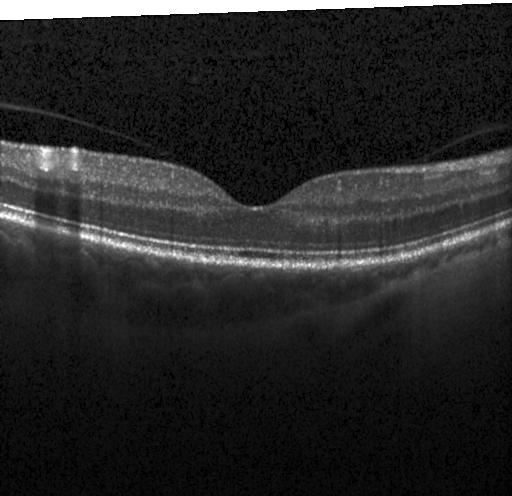 SD-OCT, optical coherence tomography B-scan, instrument: Heidelberg Spectralis. Diagnosis: neither choroidal neovascularization, diabetic macular edema, nor drusen.